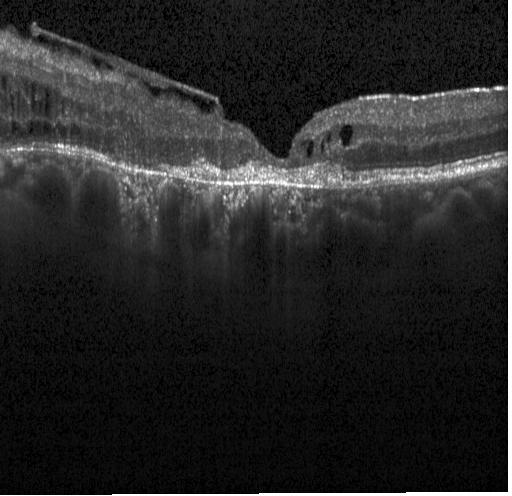
Optical coherence tomography B-scan; fovea-centered.
Finding: a choroidal neovascular membrane.